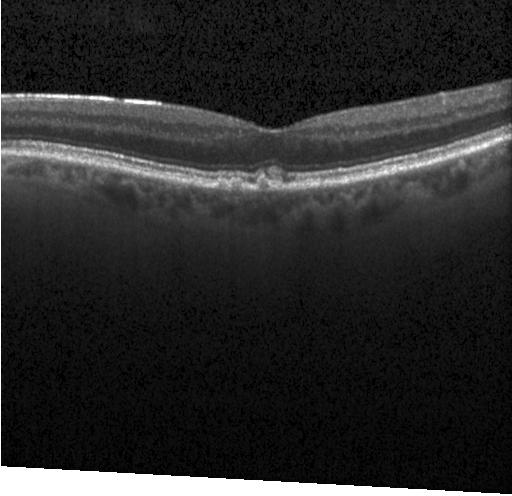
Fovea-centered. SD-OCT. OCT B-scan — This B-scan demonstrates sub-RPE drusenoid deposits.